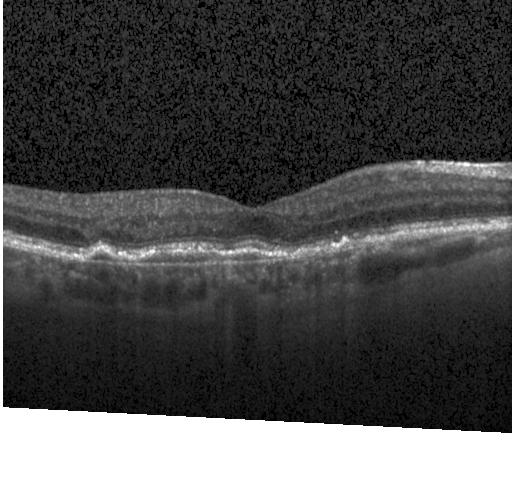
Optical coherence tomography B-scan · Heidelberg Spectralis OCT system · horizontal scan through the fovea
Finding: choroidal neovascularization.